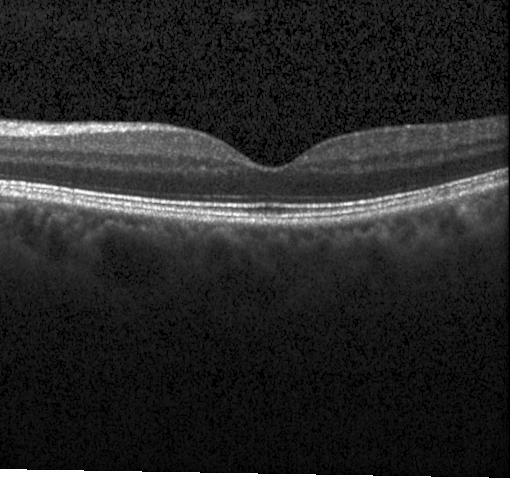

Dx: neither CNV, DME, nor drusen.